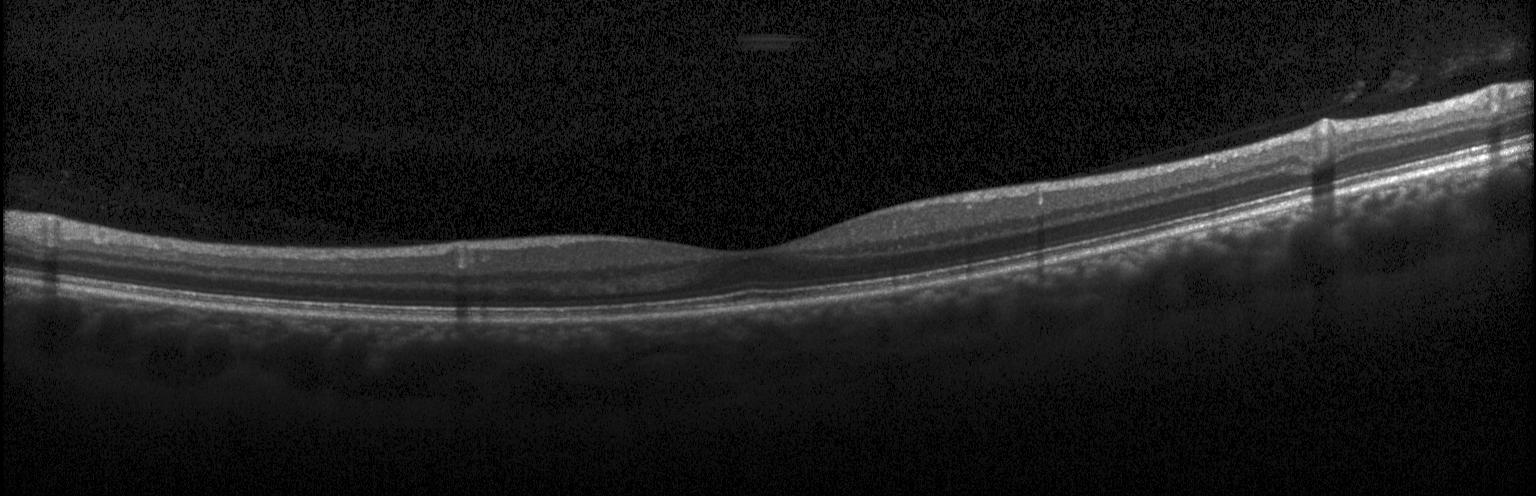 Spectral-domain optical coherence tomography · optical coherence tomography B-scan — Finding: no choroidal neovascularization, diabetic macular edema, or drusen.